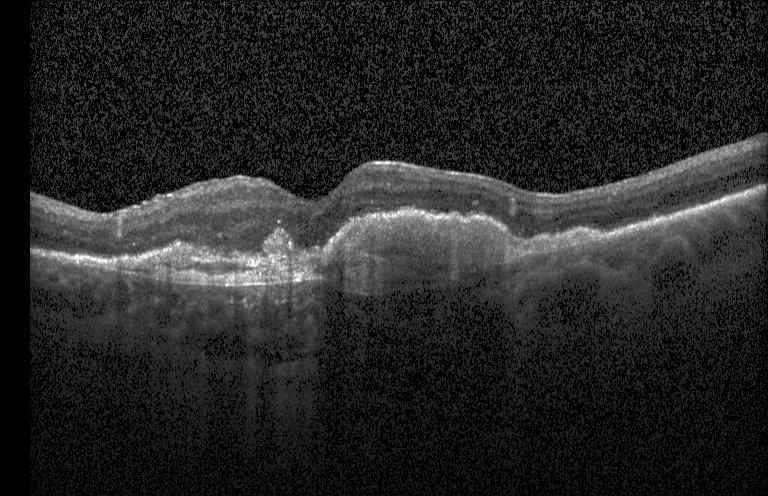
OCT line scan; instrument: Heidelberg Spectralis — Dx: a choroidal neovascular membrane.